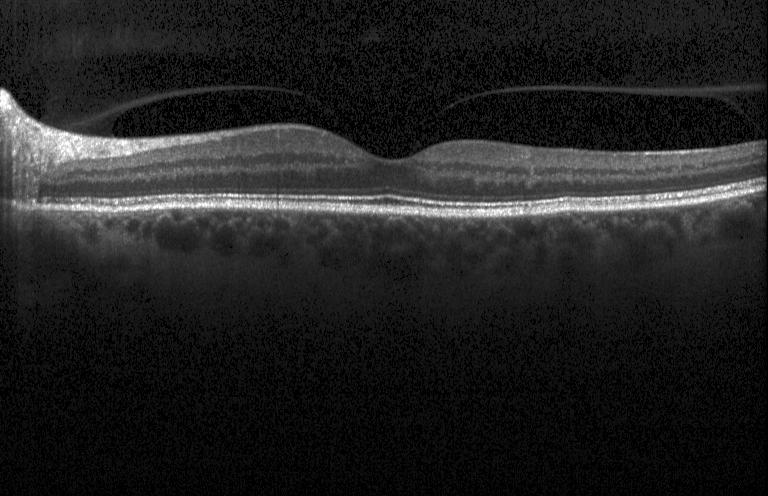 Through the macula. OCT line scan. Spectral-domain OCT — Impression: neither choroidal neovascularization, diabetic macular edema, nor drusen.